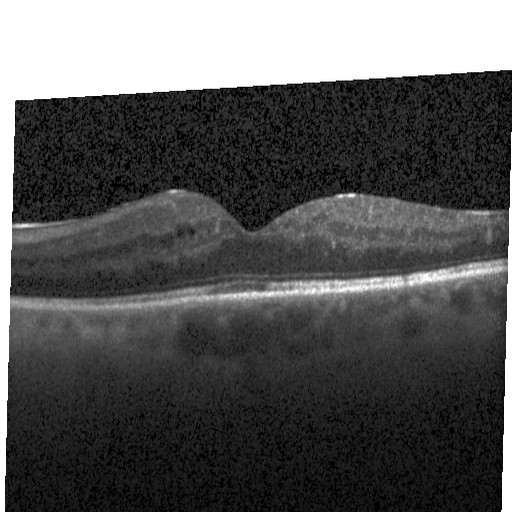

Finding: diabetic macular edema (DME).